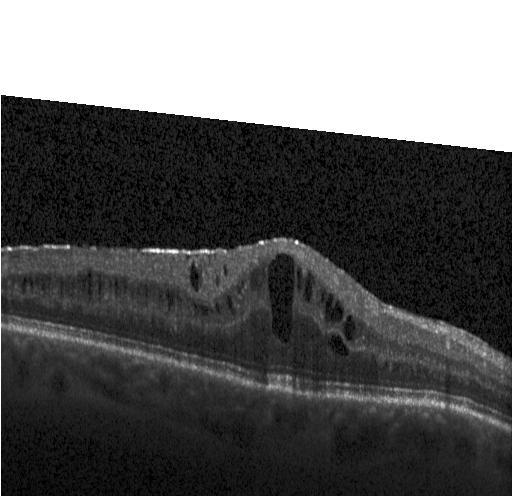

Impression: diabetic macular edema (DME).